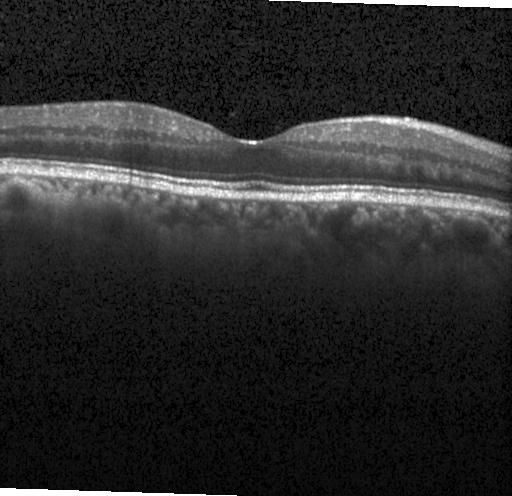
Dx: no choroidal neovascularization, diabetic macular edema, or drusen.